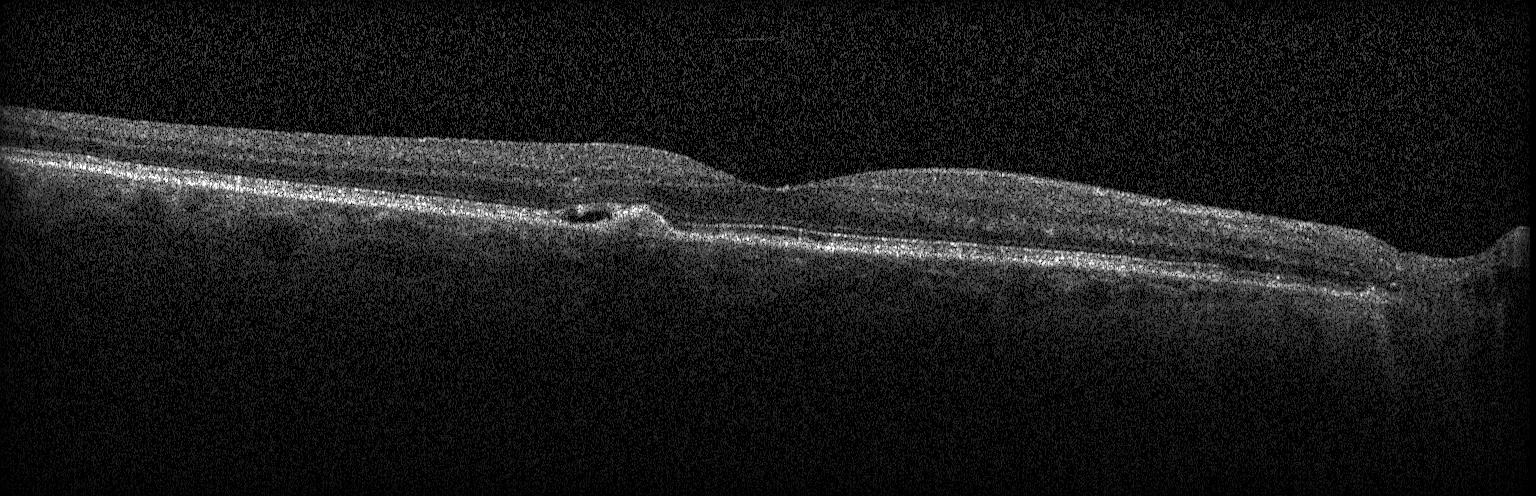
Spectral-domain OCT. Optical coherence tomography B-scan. Heidelberg Spectralis
Diagnosis: choroidal neovascularization (CNV).